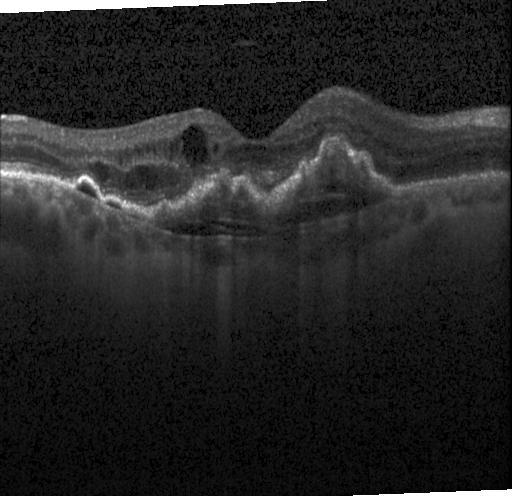 Impression: choroidal neovascularization (CNV).